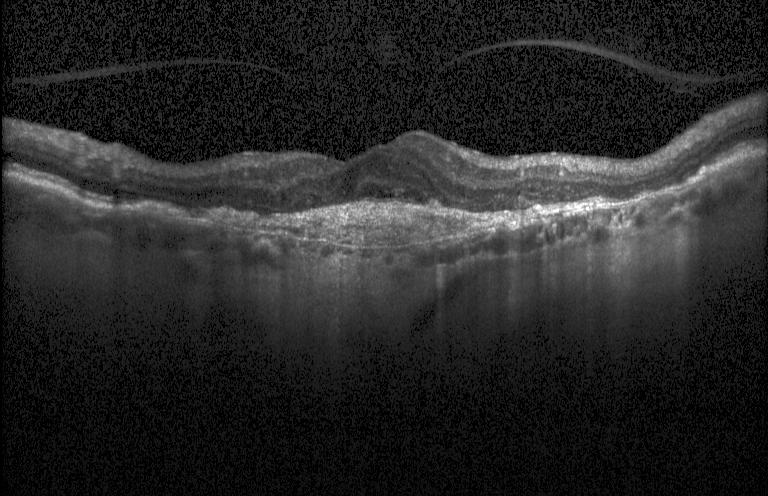

Instrument: Heidelberg Spectralis · optical coherence tomography scan · SD-OCT · fovea-centered — Macular OCT: choroidal neovascularization (CNV).